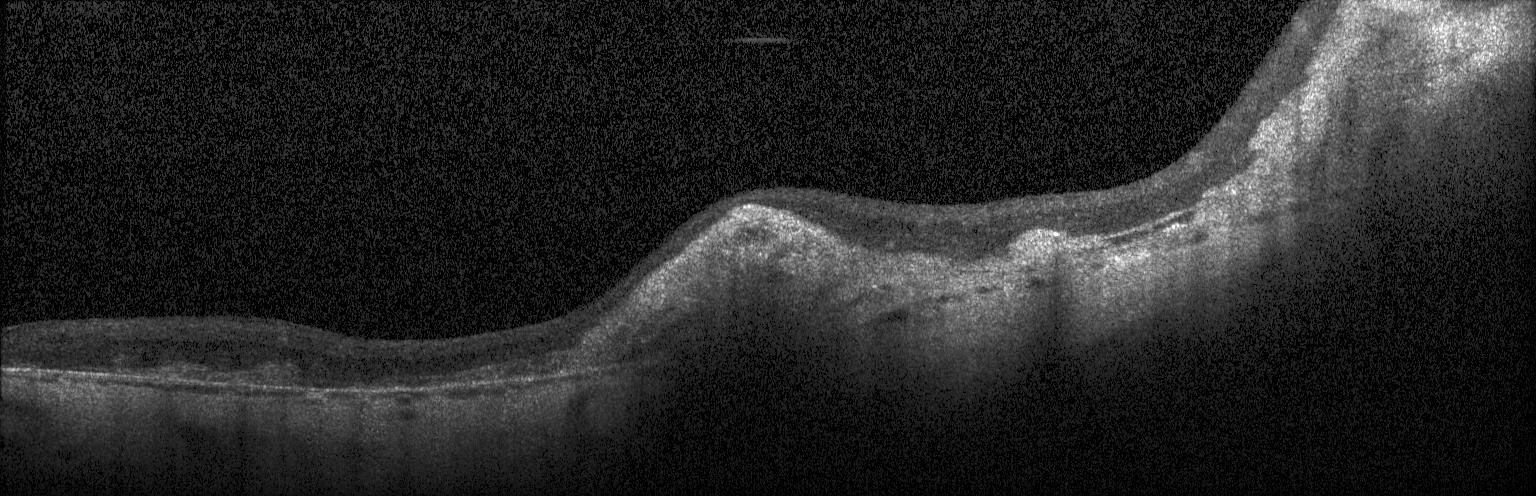

Retinal OCT B-scan. Assessment: a choroidal neovascular membrane.